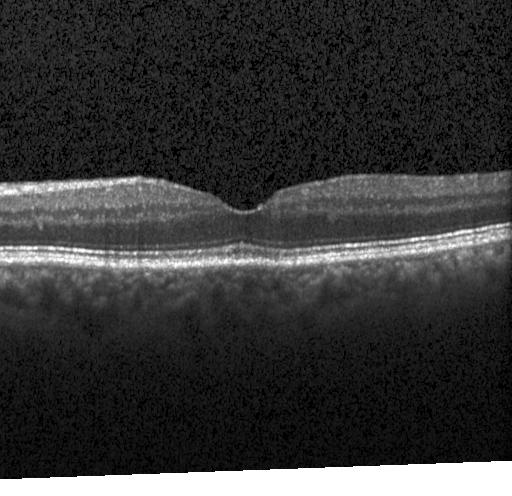
Horizontal scan through the fovea. Instrument: Heidelberg Spectralis. SD-OCT. Optical coherence tomography scan.
Assessment: no CNV, DME, or drusen.